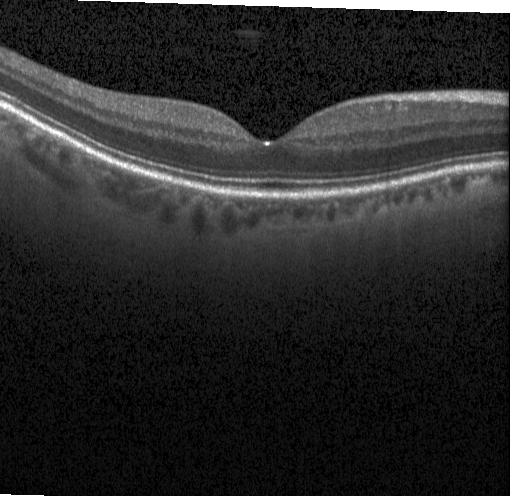 OCT B-scan; spectral-domain OCT.
Finding: neither choroidal neovascularization, diabetic macular edema, nor drusen.